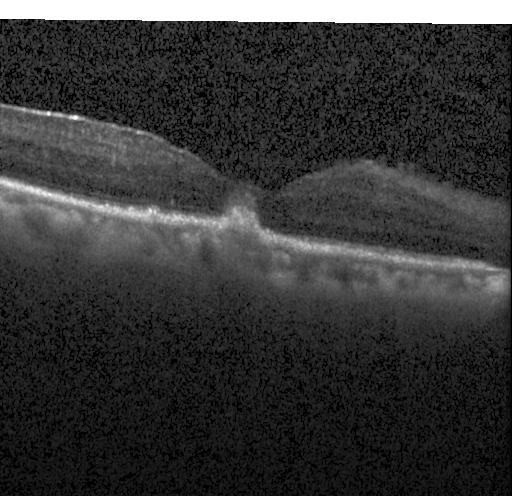 Heidelberg Spectralis, spectral-domain optical coherence tomography, retinal OCT B-scan. Finding: choroidal neovascularization.